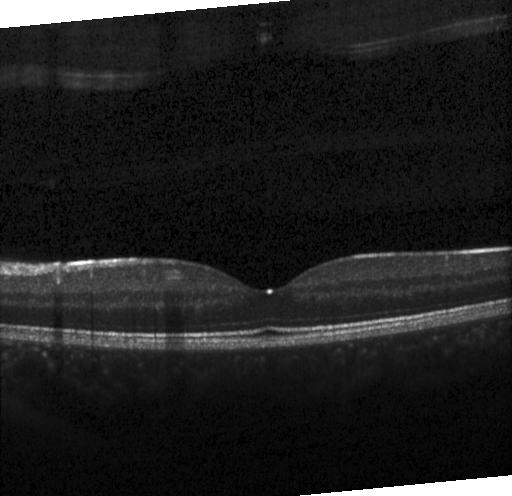 Spectral-domain optical coherence tomography · horizontal scan through the fovea · instrument: Heidelberg Spectralis · optical coherence tomography B-scan — This B-scan demonstrates no choroidal neovascularization, diabetic macular edema, or drusen.